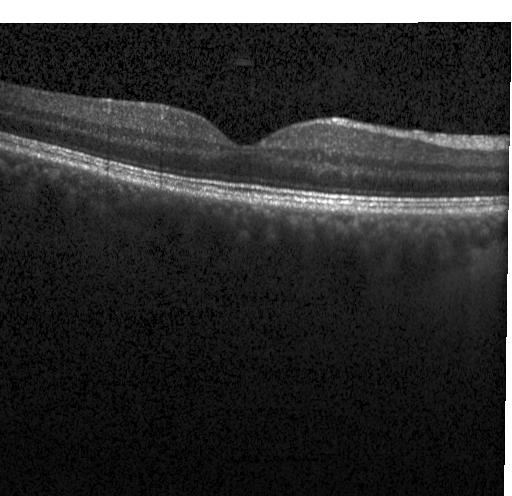

Heidelberg Spectralis OCT system, spectral-domain optical coherence tomography, through the macula, optical coherence tomography scan. No choroidal neovascularization, diabetic macular edema, or drusen.